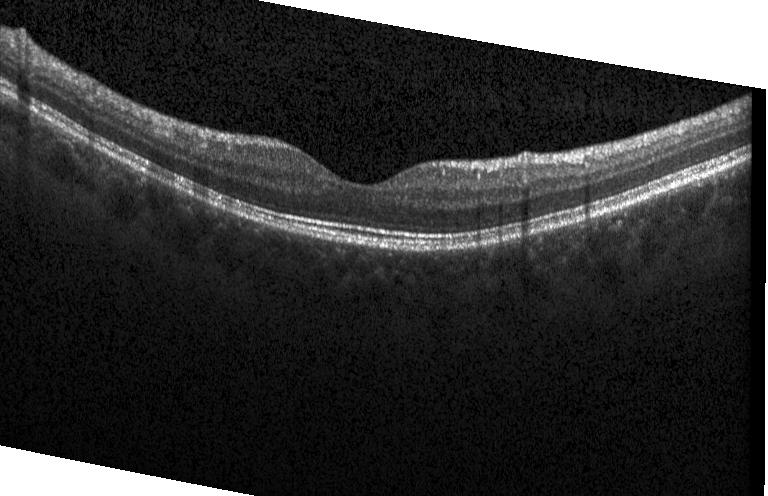
Optical coherence tomography scan
Impression: no CNV, no DME, and no drusen.